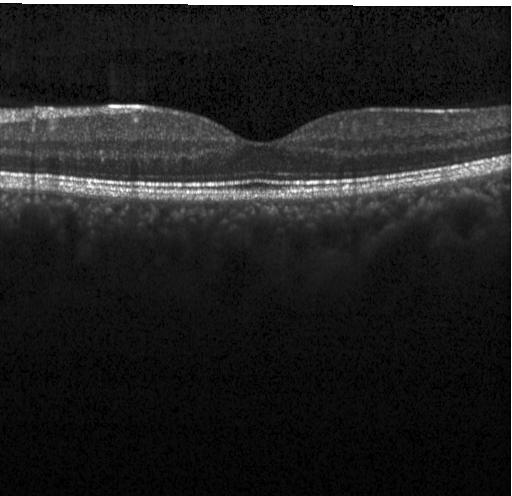
Diagnosis: no choroidal neovascularization, diabetic macular edema, or drusen.